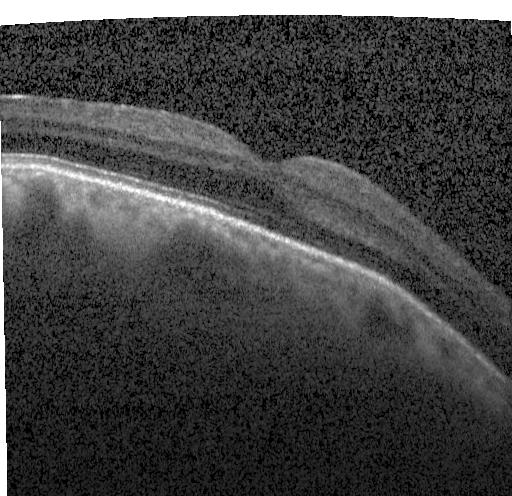
Impression: neither choroidal neovascularization, diabetic macular edema, nor drusen.